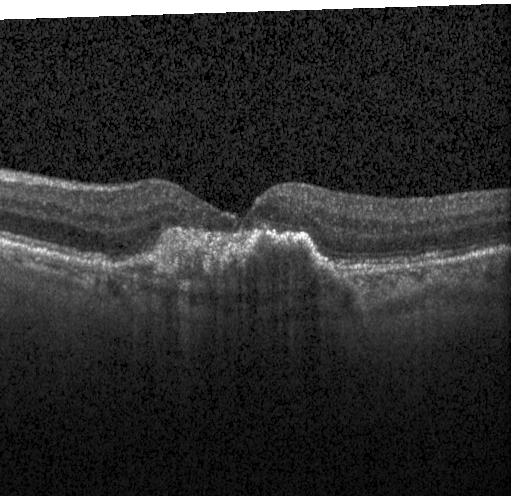 Spectral-domain OCT; optical coherence tomography scan.
Choroidal neovascularization.